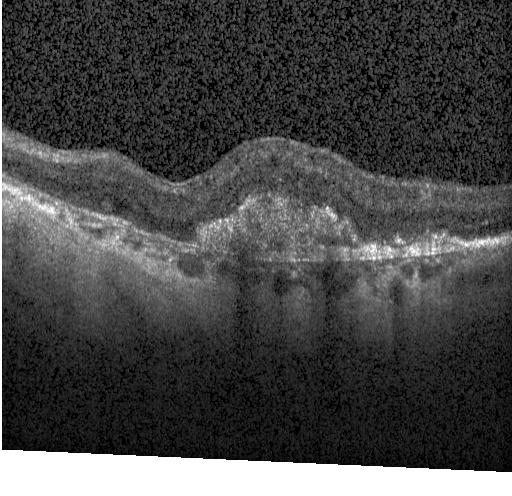 Fovea-centered, spectral-domain optical coherence tomography, retinal OCT B-scan
Finding: a choroidal neovascular membrane.